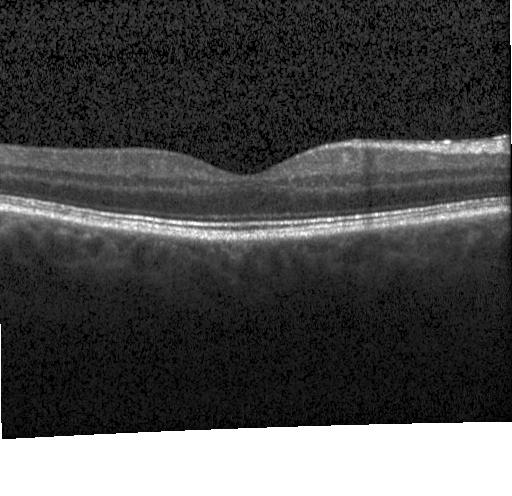 Optical coherence tomography scan · Heidelberg Spectralis · fovea-centered · spectral-domain OCT — Assessment: neither choroidal neovascularization, diabetic macular edema, nor drusen.